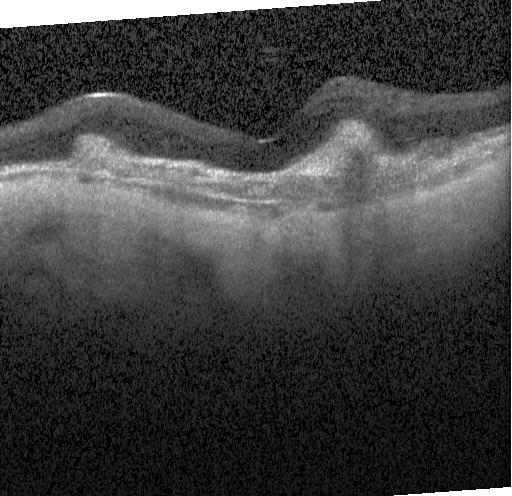
OCT line scan — This B-scan demonstrates CNV.